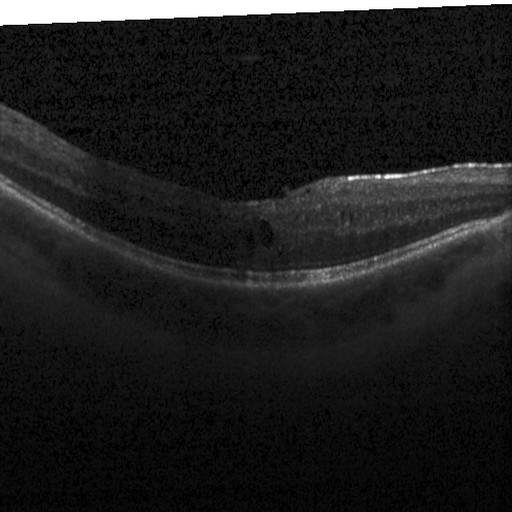 Optical coherence tomography scan · macular scan. This B-scan demonstrates DME.